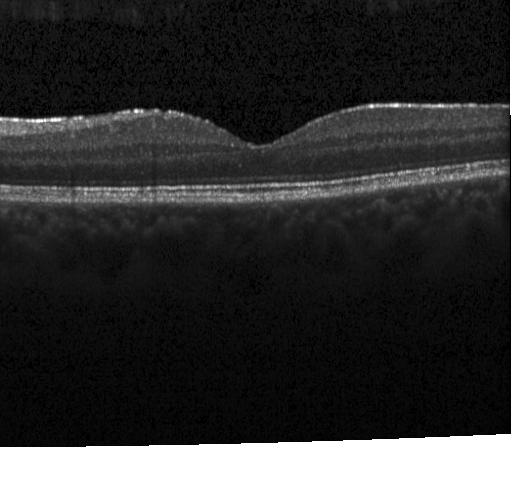

Diagnosis: no CNV, DME, or drusen.